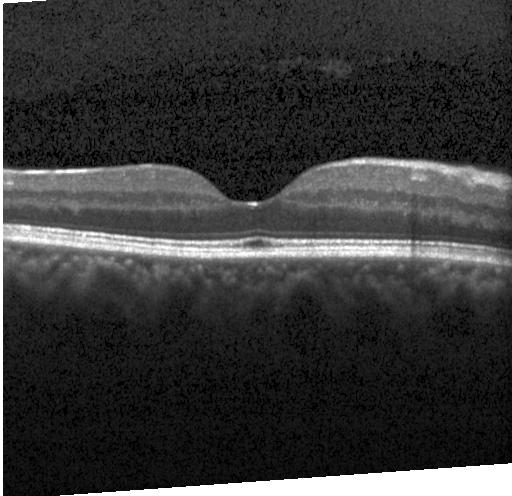 Optical coherence tomography scan, centered on the fovea, spectral-domain optical coherence tomography — Assessment: no evidence of CNV, DME, or drusen.